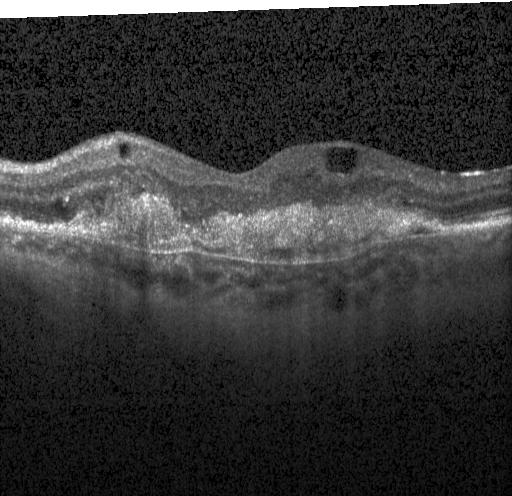
Spectral-domain optical coherence tomography; OCT B-scan.
Impression: choroidal neovascularization.